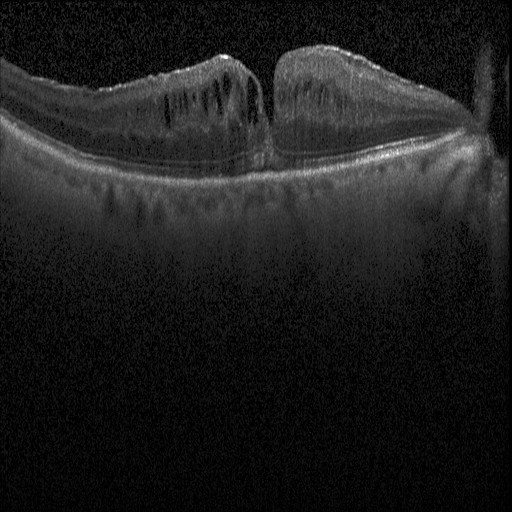 Diagnosis: diabetic macular edema (DME).